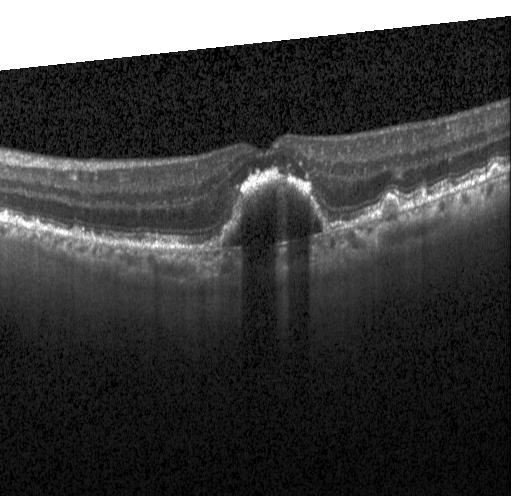 Optical coherence tomography scan; SD-OCT; macular scan. OCT finding: a choroidal neovascular membrane.